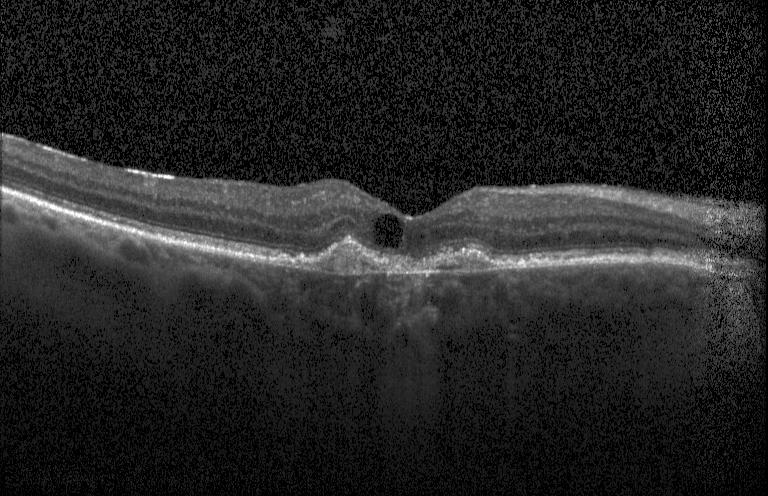 Retinal OCT cross-section. Assessment: choroidal neovascularization (CNV).